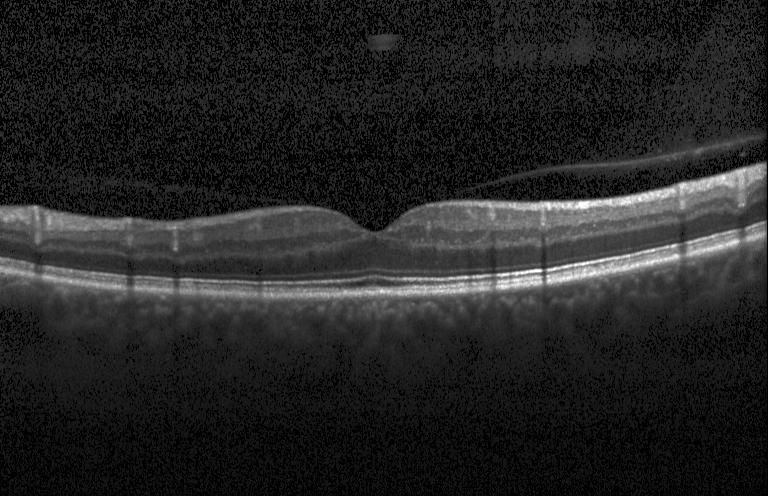
No CNV, DME, or drusen.